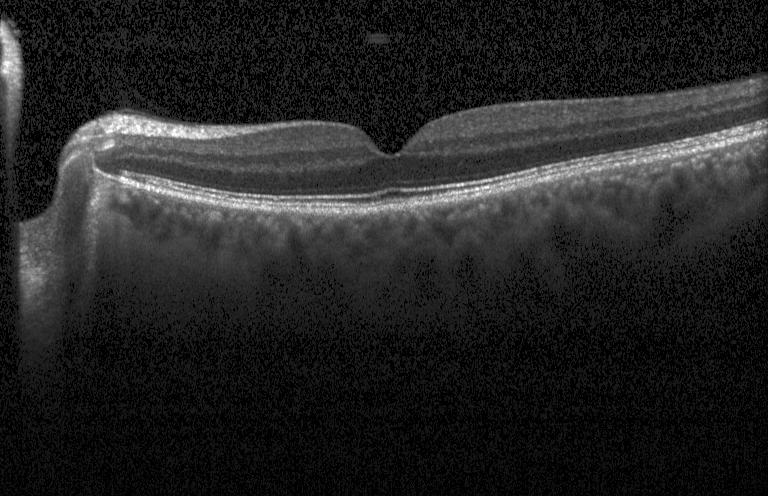
Optical coherence tomography B-scan. SD-OCT. Impression: no choroidal neovascularization, no diabetic macular edema, and no drusen.